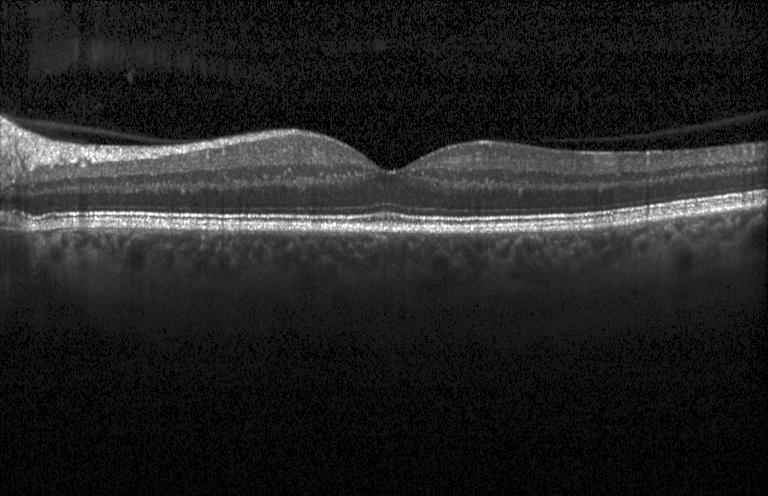 Spectral-domain optical coherence tomography. Retinal OCT cross-section. Macular scan.
Finding: no evidence of choroidal neovascularization, diabetic macular edema, or drusen.